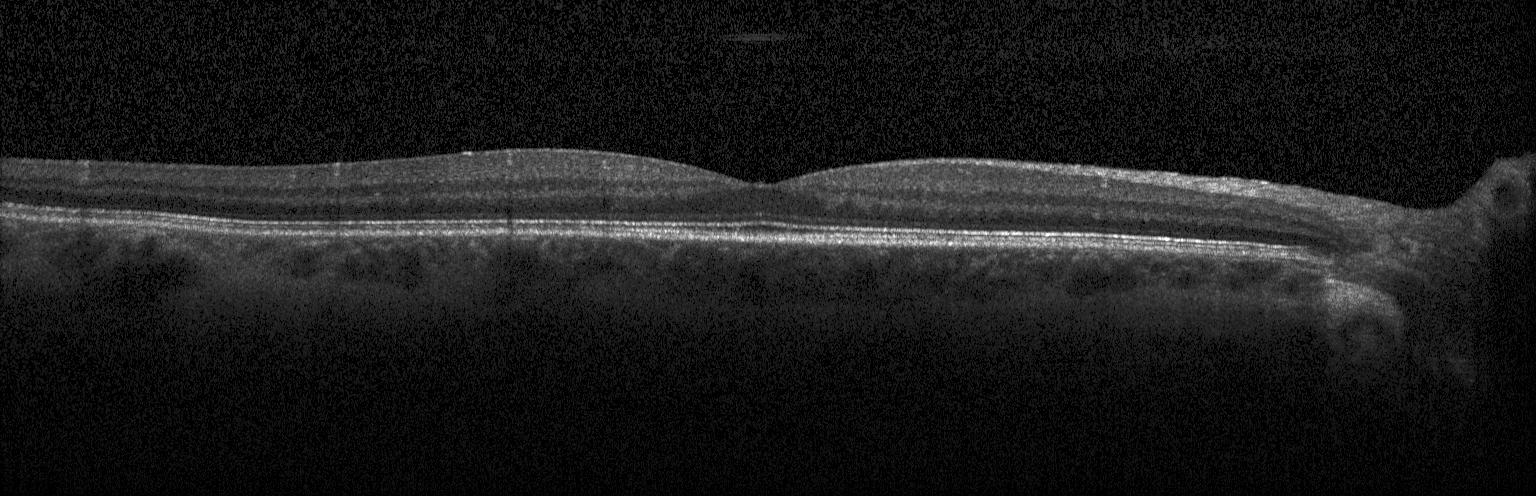 Macular OCT demonstrating no choroidal neovascularization, diabetic macular edema, or drusen.